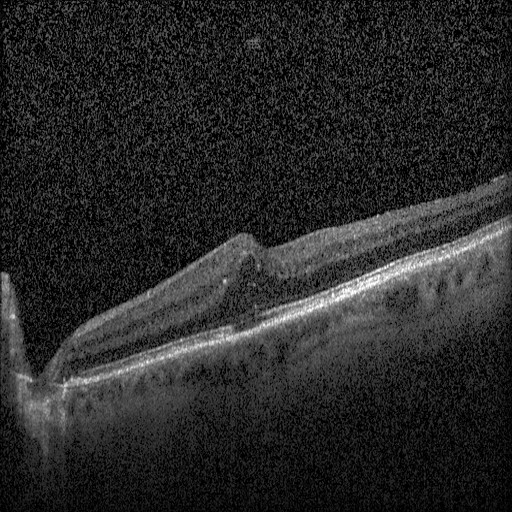

Retinal OCT cross-section. Diagnosis: DME.